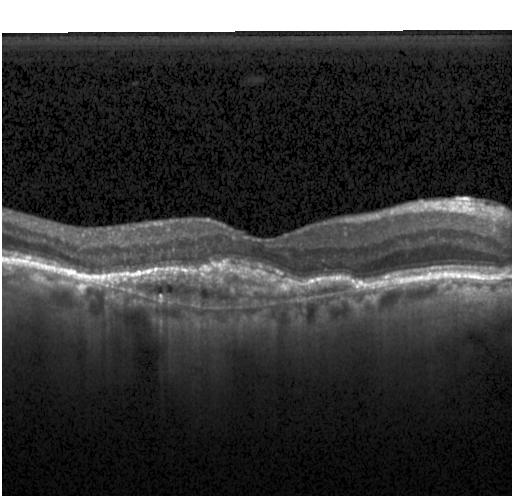
Optical coherence tomography B-scan · fovea-centered · spectral-domain OCT · Heidelberg Spectralis. Diagnosis: choroidal neovascularization (CNV).